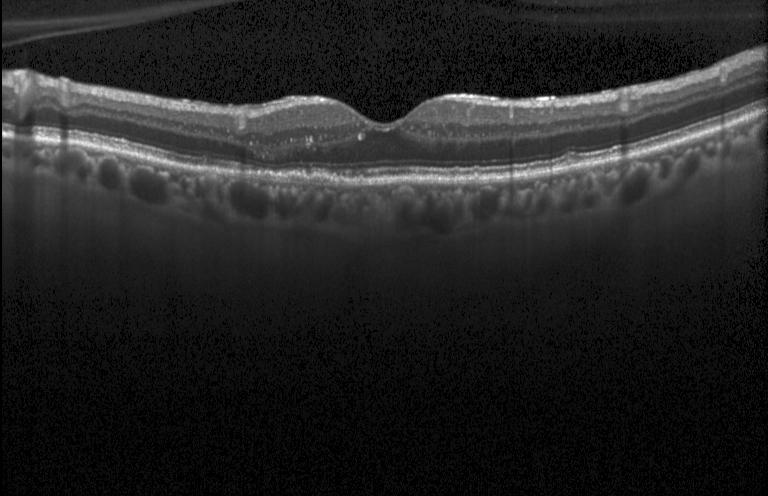 Retinal OCT cross-section, SD-OCT
Macular OCT: multiple drusen.